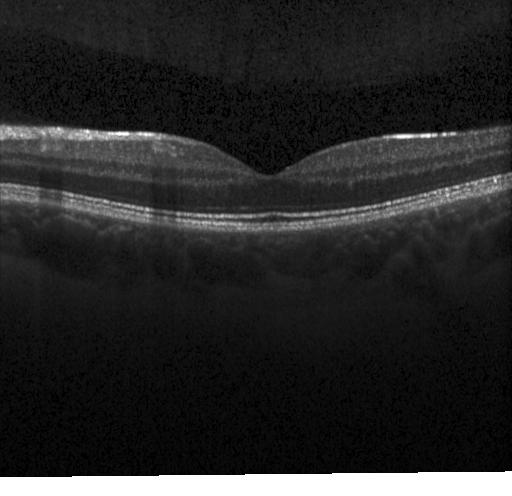 Diagnosis: no evidence of CNV, DME, or drusen.